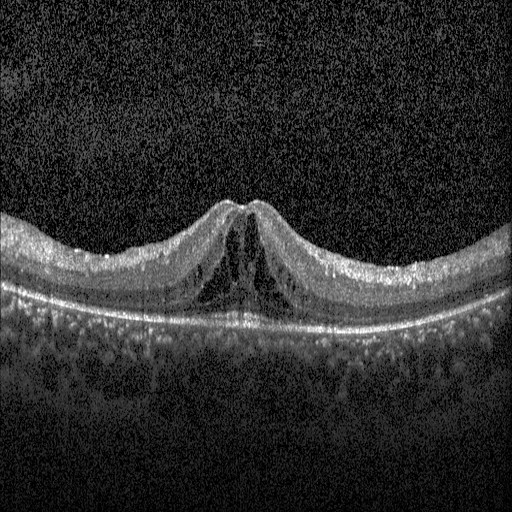 Optical coherence tomography scan · spectral-domain optical coherence tomography · macular scan · acquired on a Heidelberg Spectralis. Finding: diabetic macular edema.